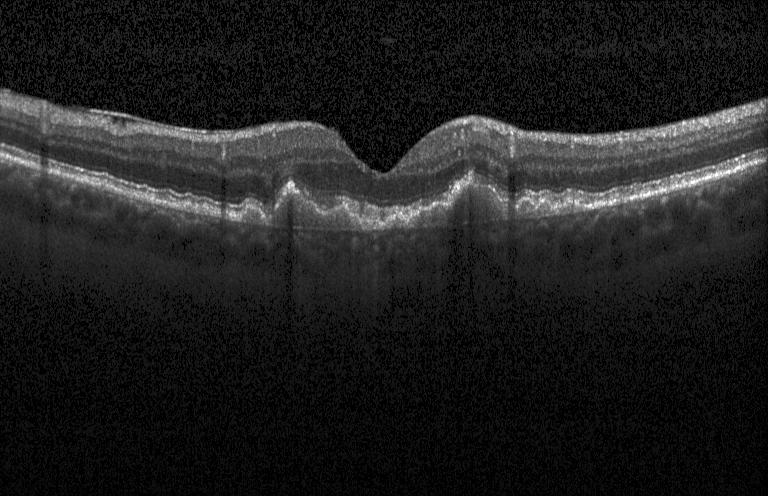
Dx: multiple drusen.